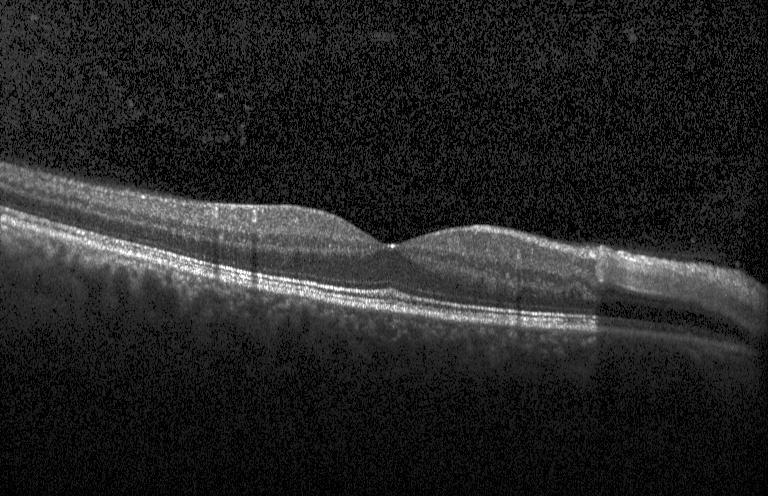 Retinal OCT cross-section; acquired on a Heidelberg Spectralis — No choroidal neovascularization, diabetic macular edema, or drusen.